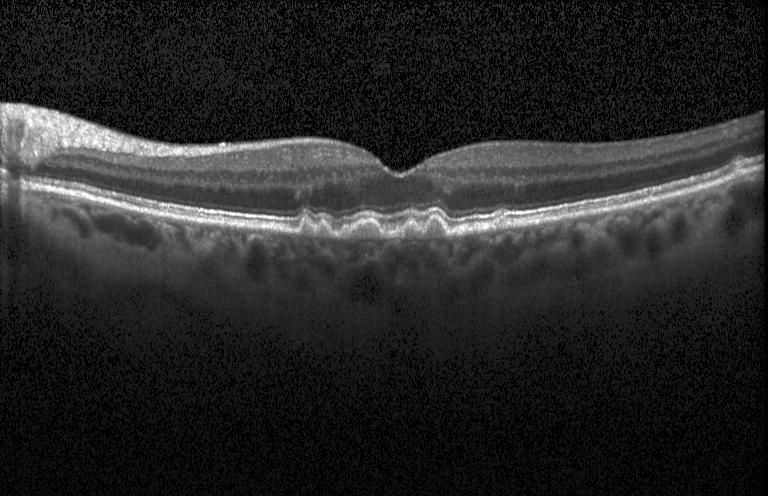 Impression: drusen.